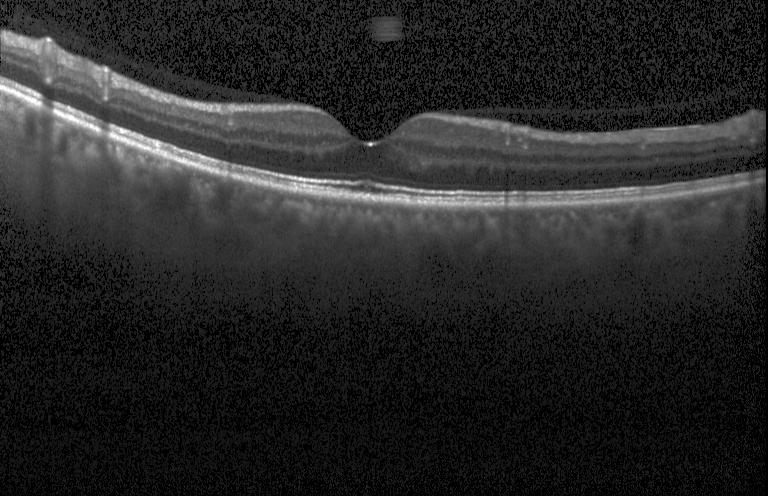

Impression: neither CNV, DME, nor drusen.